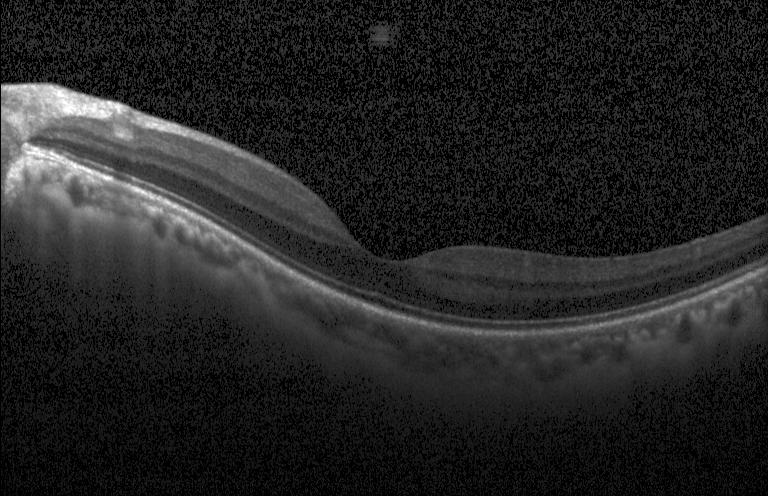
Spectral-domain optical coherence tomography · retinal OCT cross-section · horizontal scan through the fovea · instrument: Heidelberg Spectralis
Impression: no choroidal neovascularization, no diabetic macular edema, and no drusen.